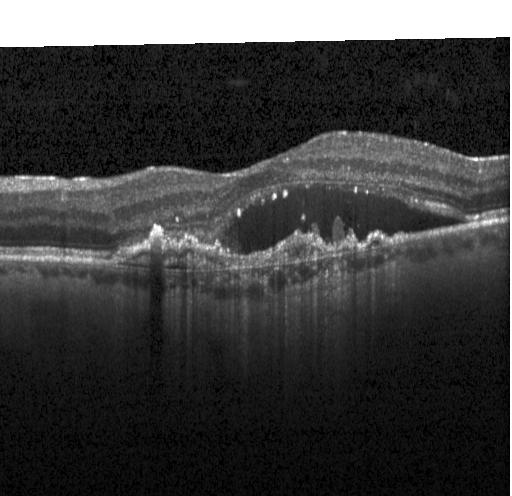

Impression: a choroidal neovascular membrane.